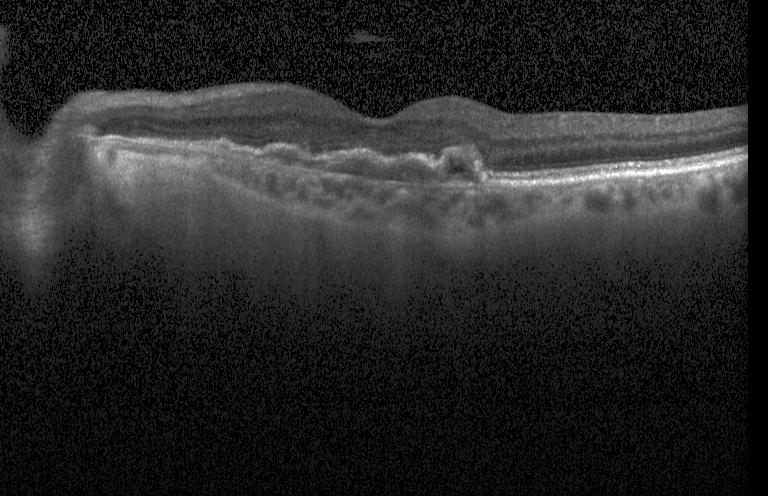 Fovea-centered, spectral-domain optical coherence tomography, Heidelberg Spectralis OCT system, OCT line scan
Assessment: choroidal neovascularization.